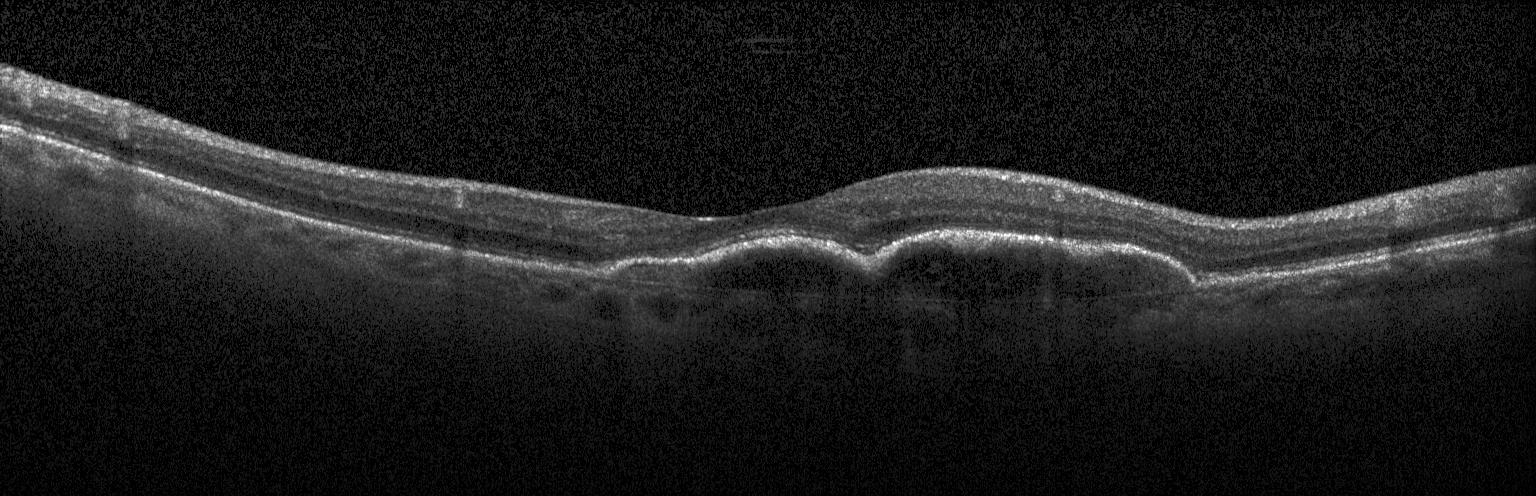

Retinal OCT cross-section.
Finding: CNV.